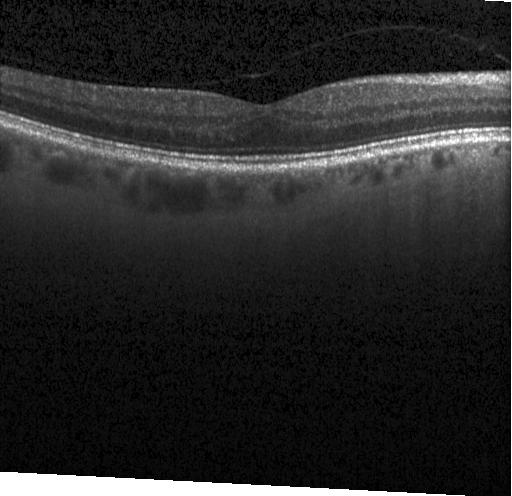

Centered on the fovea · SD-OCT · retinal OCT cross-section.
Finding: no CNV, DME, or drusen.